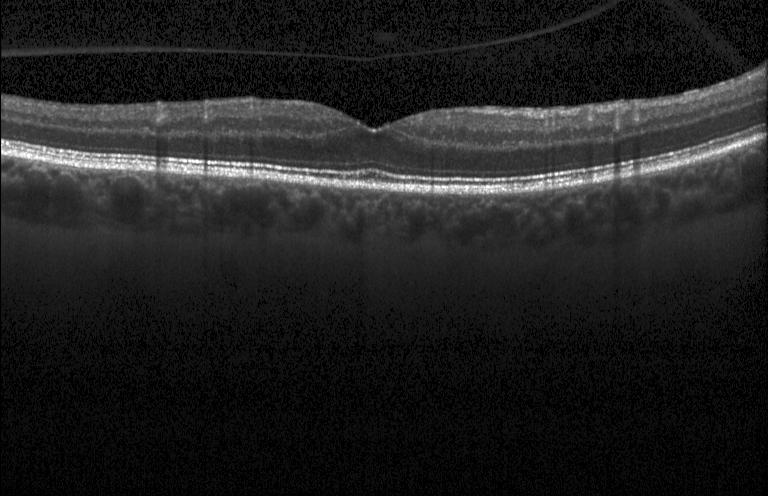 OCT line scan
Impression: no choroidal neovascularization, diabetic macular edema, or drusen.